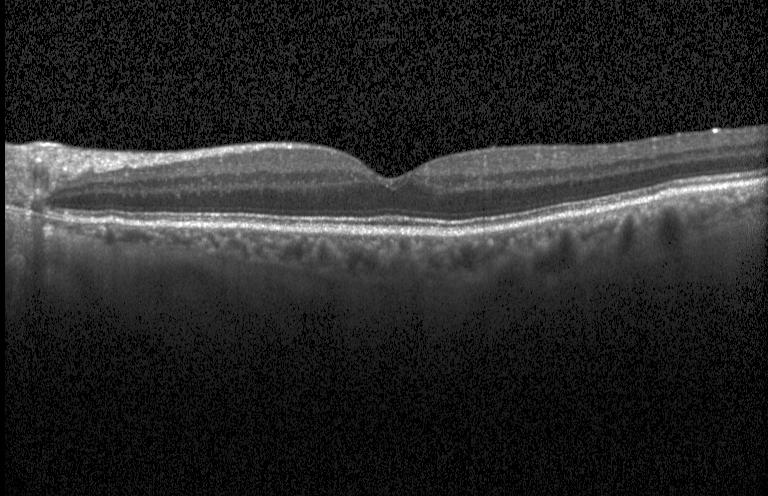

Spectral-domain optical coherence tomography. OCT line scan. Instrument: Heidelberg Spectralis.
Diagnosis: no choroidal neovascularization, no diabetic macular edema, and no drusen.